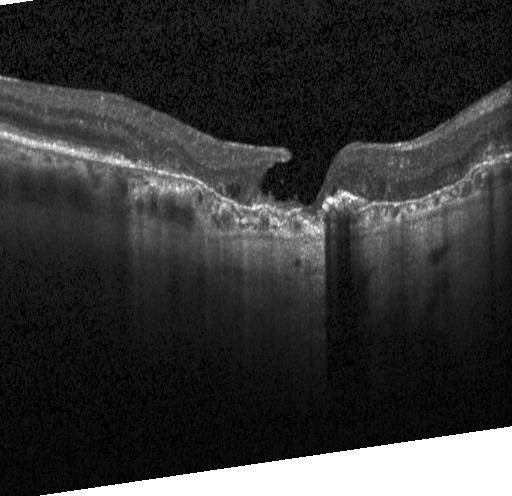

Assessment: choroidal neovascularization (CNV).